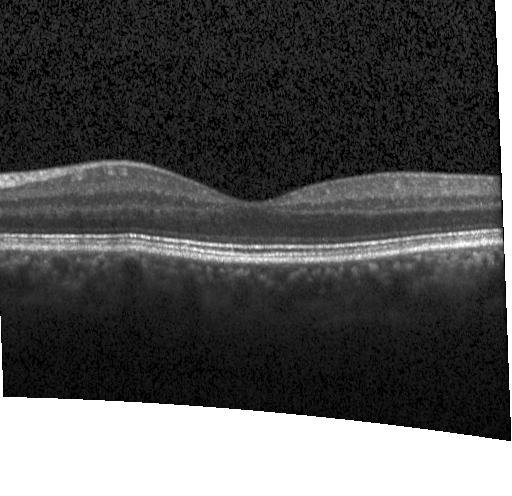
OCT B-scan.
Impression: no evidence of choroidal neovascularization, diabetic macular edema, or drusen.